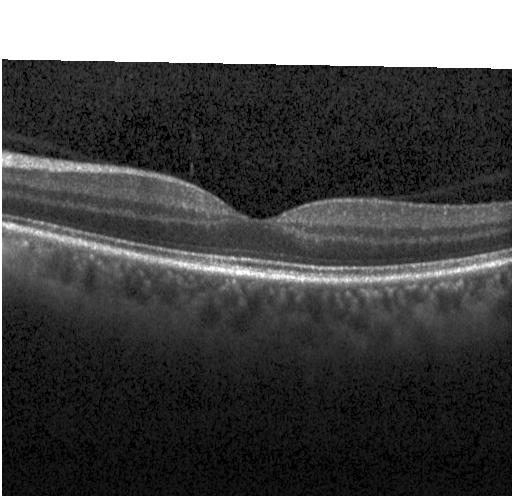
OCT scan showing neither choroidal neovascularization, diabetic macular edema, nor drusen.